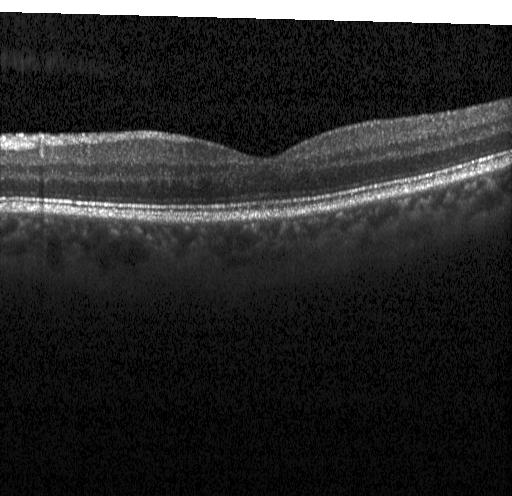
Optical coherence tomography B-scan — Dx: neither choroidal neovascularization, diabetic macular edema, nor drusen.